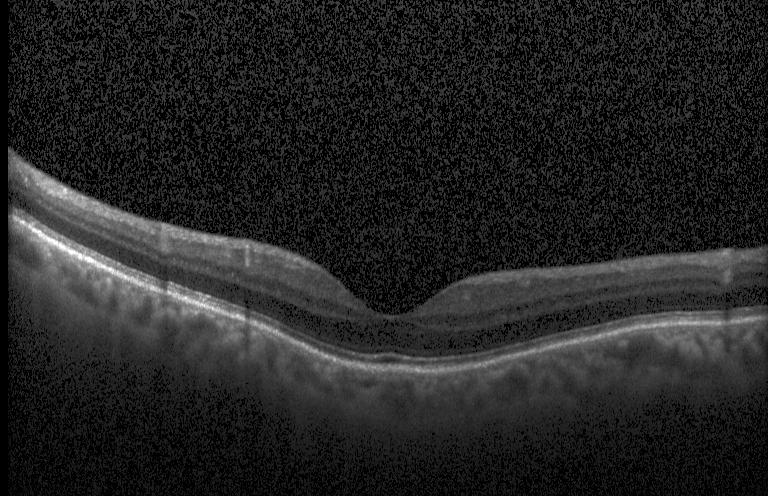
Fovea-centered · OCT line scan — Impression: neither choroidal neovascularization, diabetic macular edema, nor drusen.